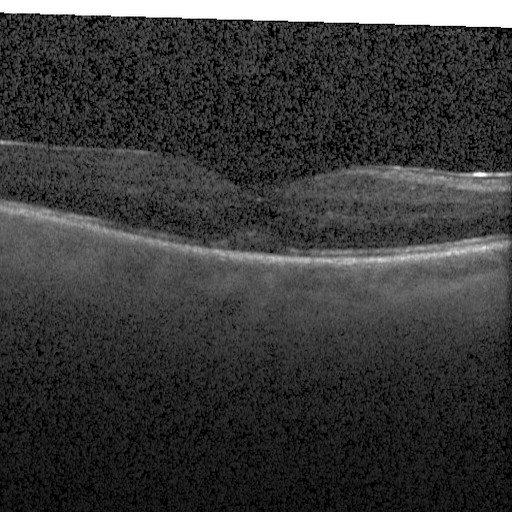
OCT line scan · SD-OCT
This B-scan demonstrates diabetic macular edema.